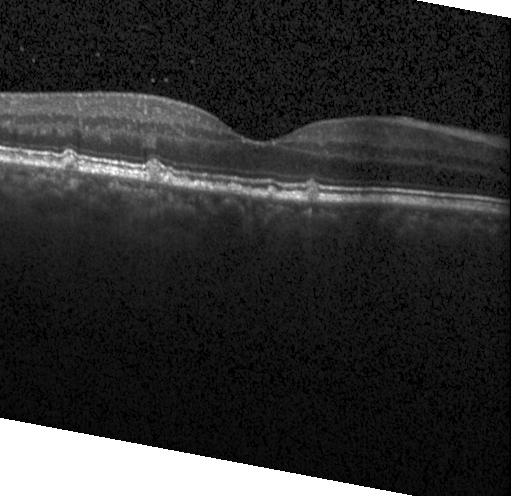
SD-OCT, optical coherence tomography scan, macular scan
Finding: drusen.